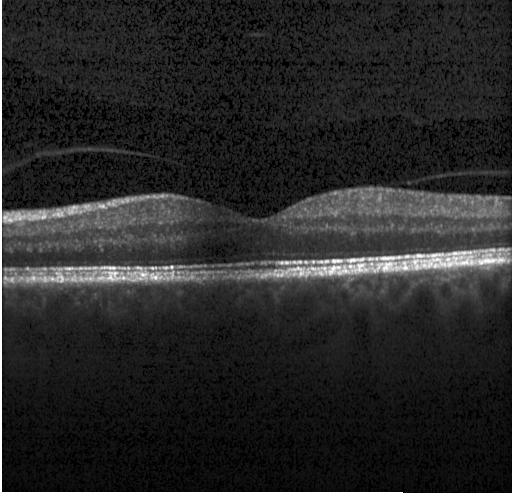

Optical coherence tomography scan
Assessment: neither choroidal neovascularization, diabetic macular edema, nor drusen.